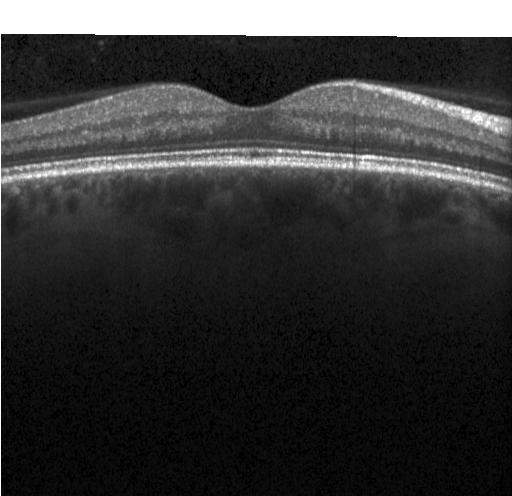 OCT line scan. Diagnosis: no choroidal neovascularization, diabetic macular edema, or drusen.